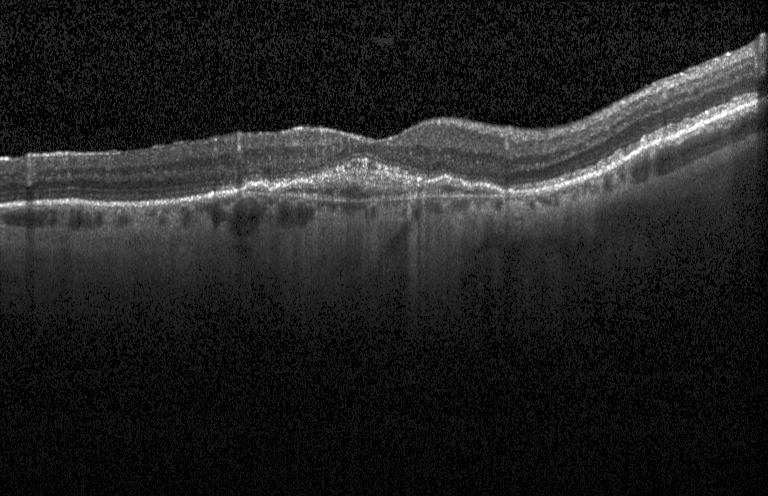
Optical coherence tomography scan. Spectral-domain optical coherence tomography.
Impression: choroidal neovascularization (CNV).